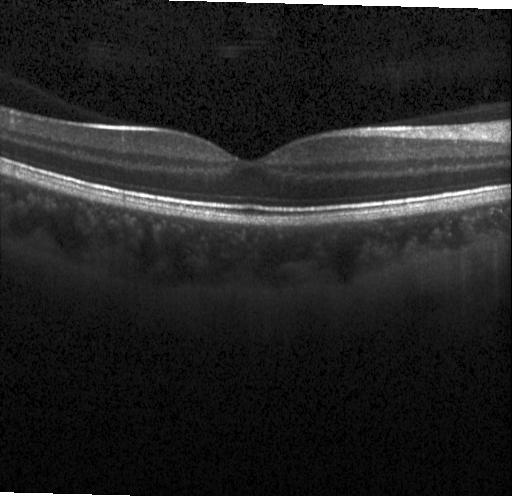
Finding: no evidence of choroidal neovascularization, diabetic macular edema, or drusen.